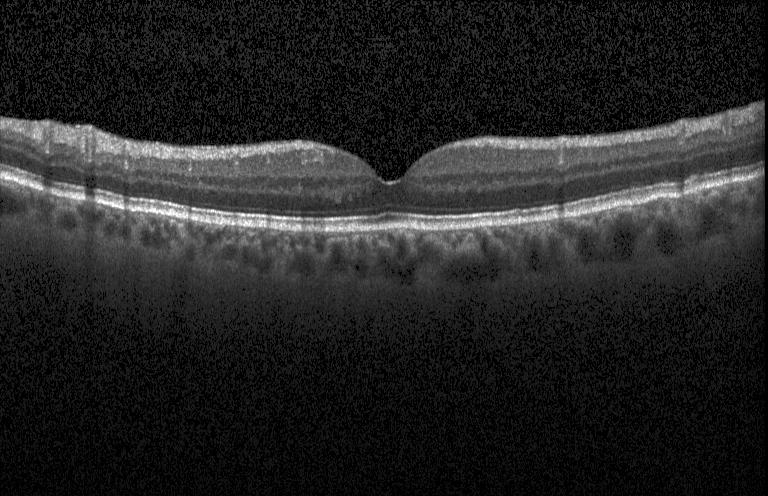

OCT finding: no evidence of choroidal neovascularization, diabetic macular edema, or drusen.